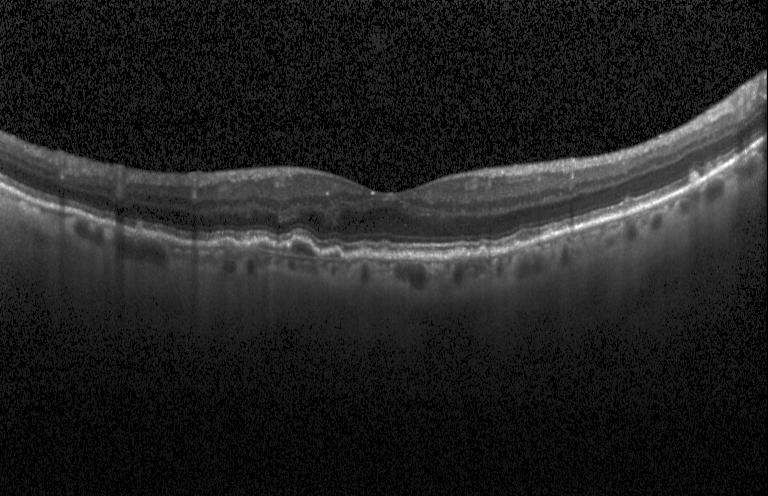
Heidelberg Spectralis OCT system · optical coherence tomography scan
Impression: drusen.